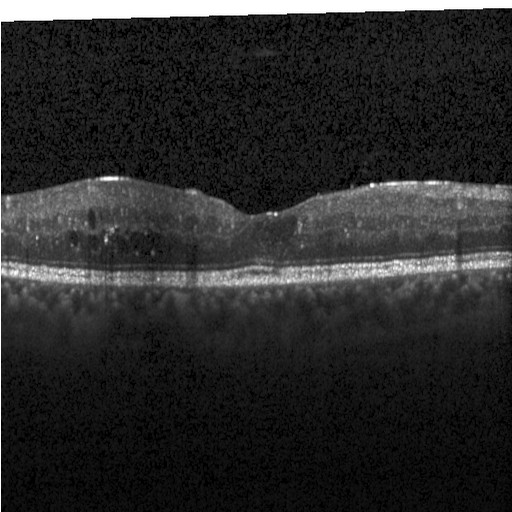

OCT B-scan; through the macula.
Impression: DME.